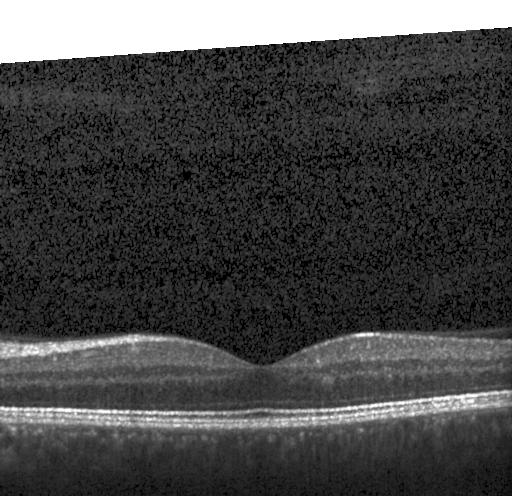
OCT B-scan showing no choroidal neovascularization, no diabetic macular edema, and no drusen.